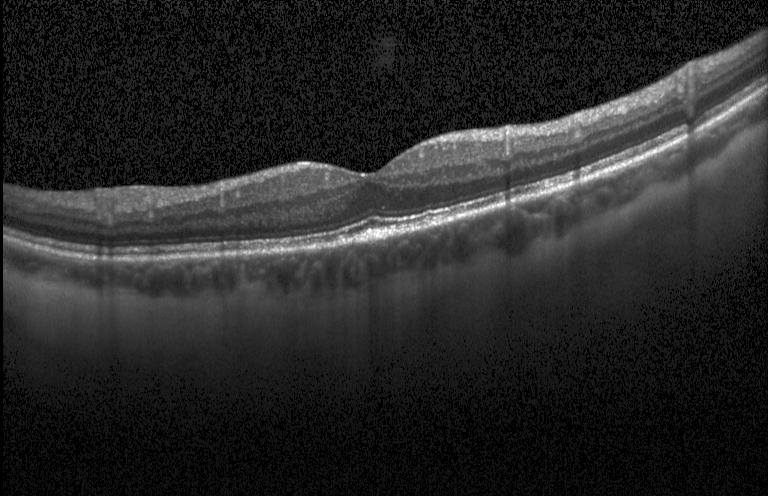
Optical coherence tomography scan — OCT finding: no evidence of CNV, DME, or drusen.